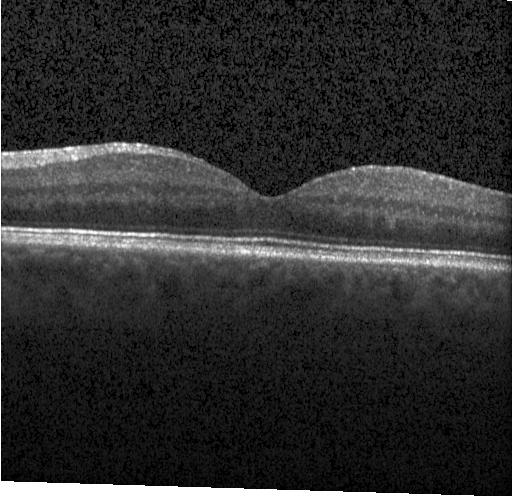

Impression: no evidence of choroidal neovascularization, diabetic macular edema, or drusen.